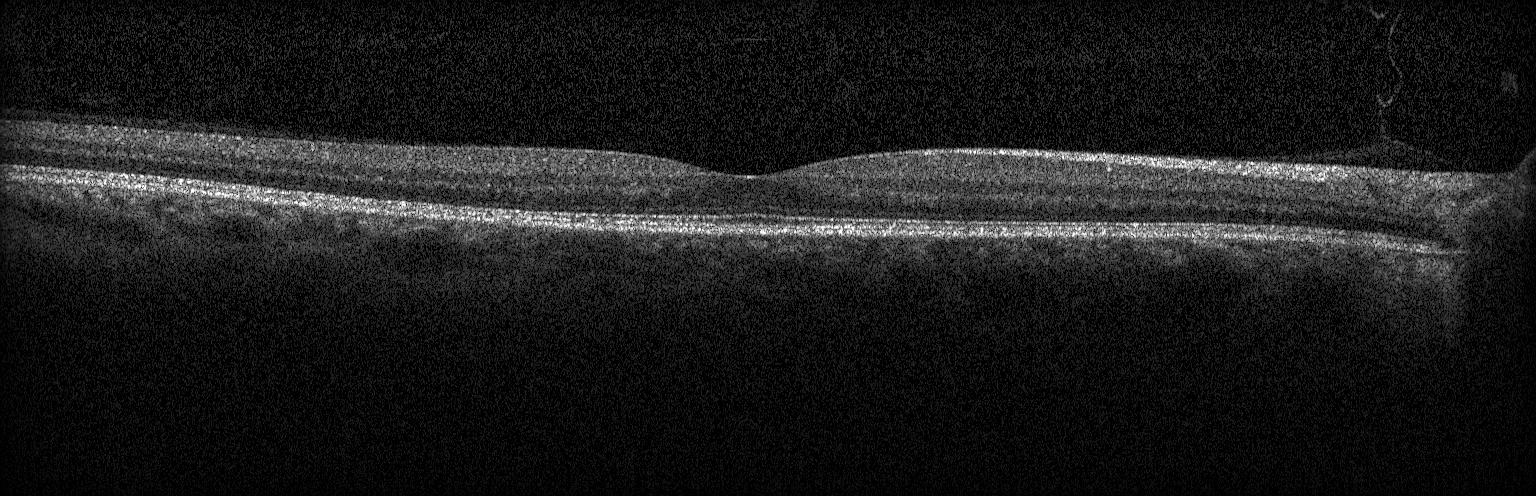

Spectral-domain optical coherence tomography. Optical coherence tomography B-scan. Centered on the fovea. Heidelberg Spectralis.
Impression: neither choroidal neovascularization, diabetic macular edema, nor drusen.